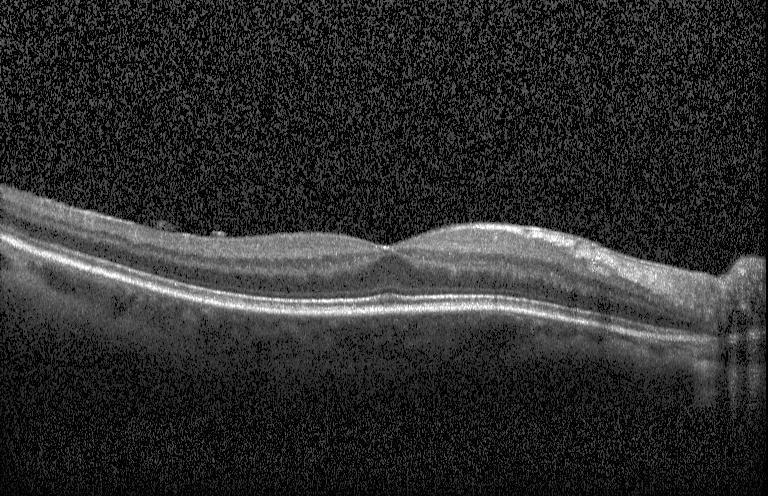

Macular OCT: no evidence of choroidal neovascularization, diabetic macular edema, or drusen.